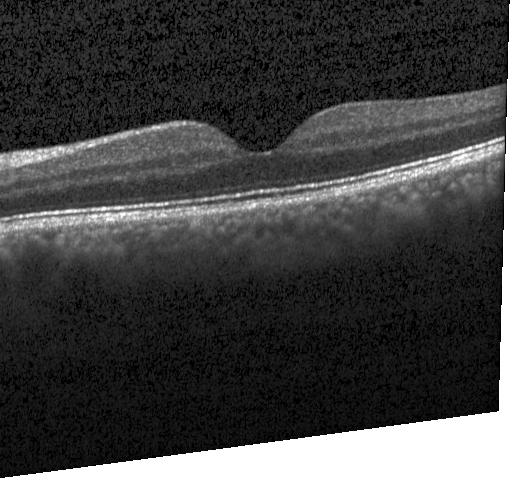

Retinal OCT cross-section — The scan shows no evidence of choroidal neovascularization, diabetic macular edema, or drusen.